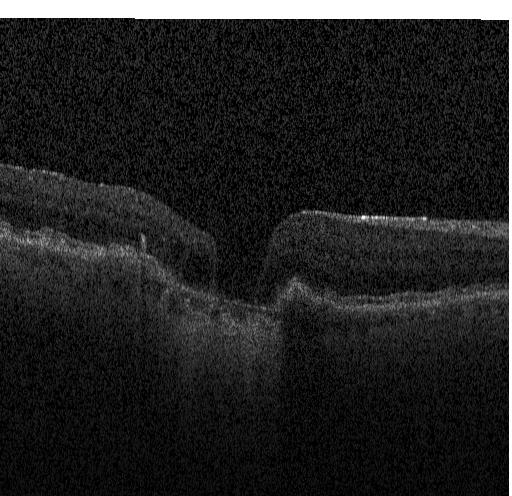
SD-OCT, fovea-centered, instrument: Heidelberg Spectralis, optical coherence tomography scan.
OCT finding: a choroidal neovascular membrane.